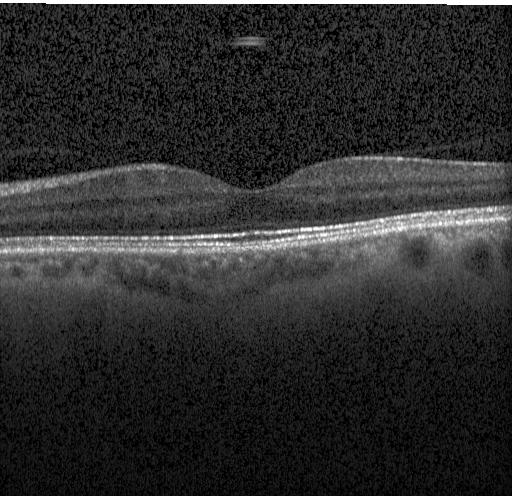

OCT finding: neither choroidal neovascularization, diabetic macular edema, nor drusen.